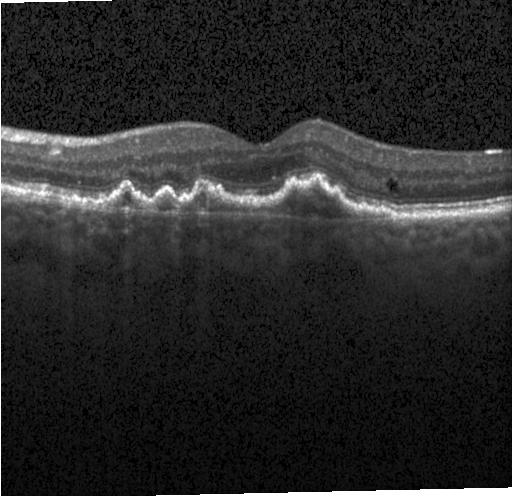

Spectral-domain optical coherence tomography; retinal OCT cross-section; macular scan
Impression: choroidal neovascularization.